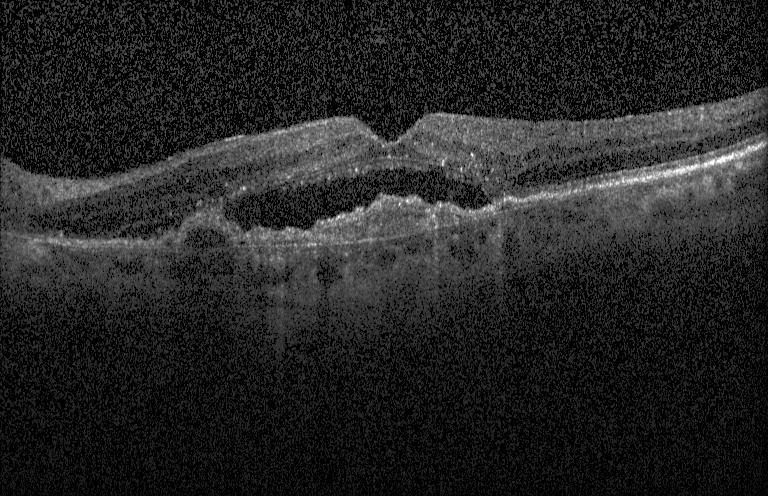 OCT B-scan.
The scan shows choroidal neovascularization.